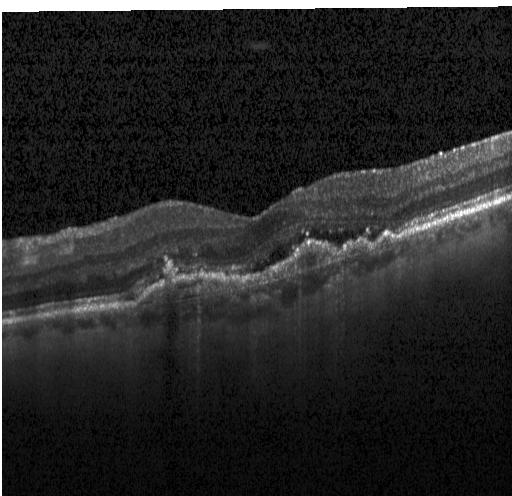
Optical coherence tomography B-scan, horizontal scan through the fovea, instrument: Heidelberg Spectralis — This B-scan demonstrates CNV.